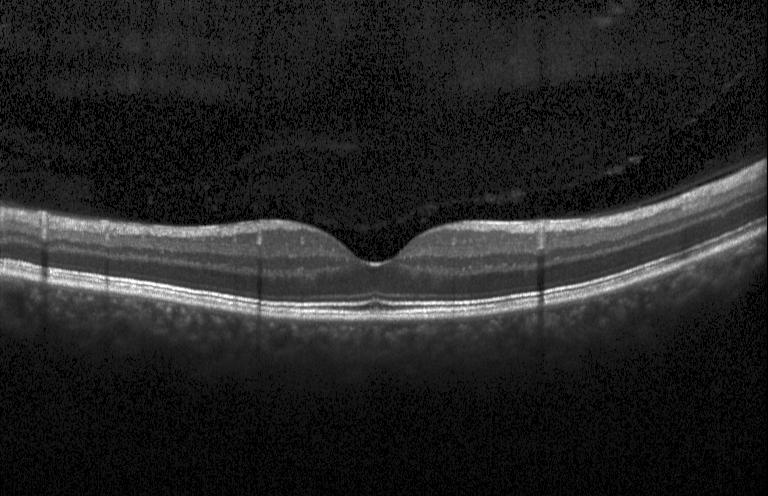

OCT scan showing neither CNV, DME, nor drusen.